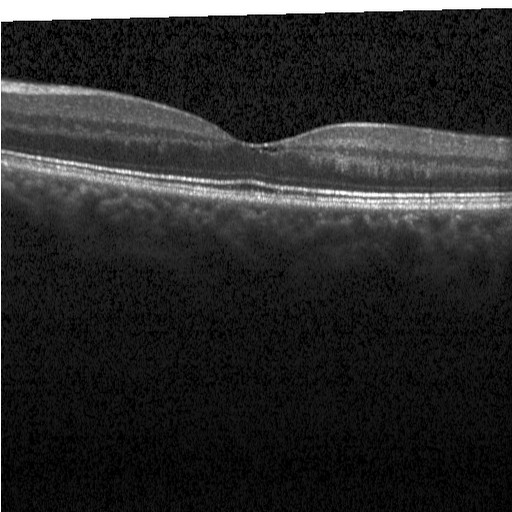
Horizontal scan through the fovea · SD-OCT · retinal OCT cross-section.
OCT finding: diabetic macular edema.